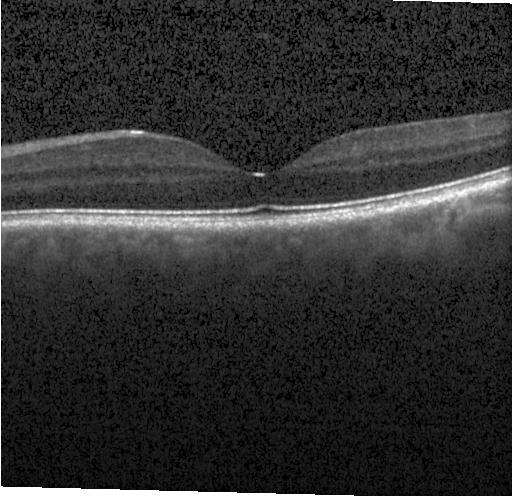 Retinal OCT cross-section.
Macular OCT: no choroidal neovascularization, no diabetic macular edema, and no drusen.